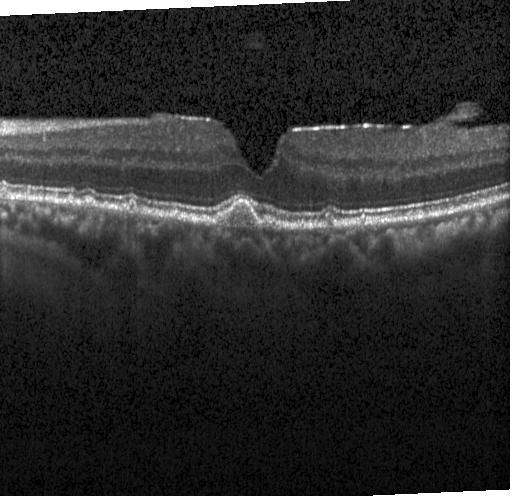
Through the macula, Heidelberg Spectralis OCT system, spectral-domain optical coherence tomography, retinal OCT B-scan.
Impression: multiple drusen.